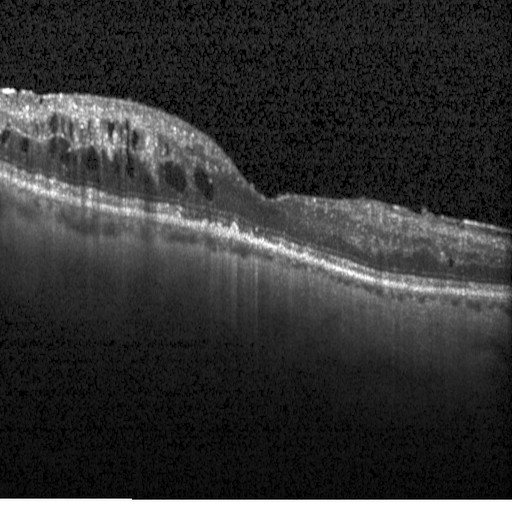

Retinal OCT cross-section showing DME.